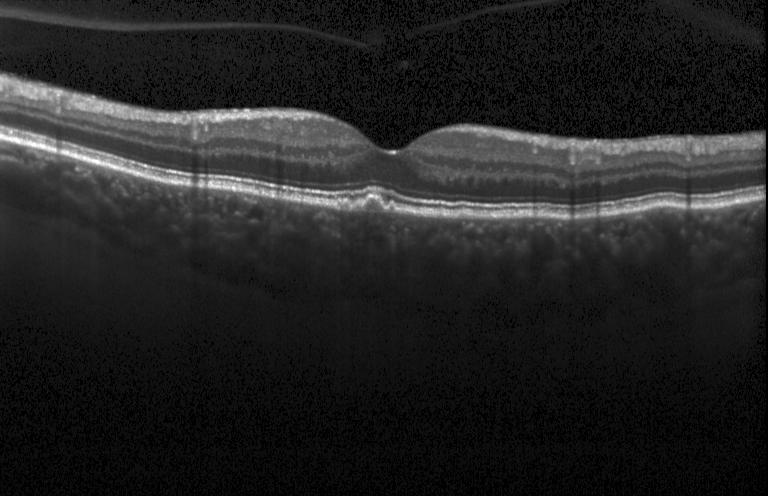

Optical coherence tomography B-scan
Diagnosis: multiple drusen.